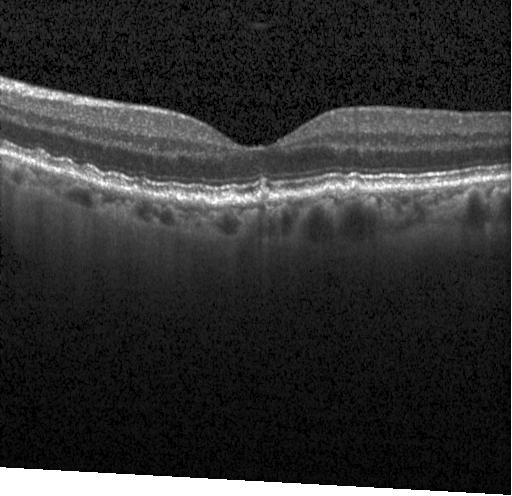
Acquired on a Heidelberg Spectralis · optical coherence tomography B-scan · spectral-domain optical coherence tomography. This B-scan demonstrates drusen.